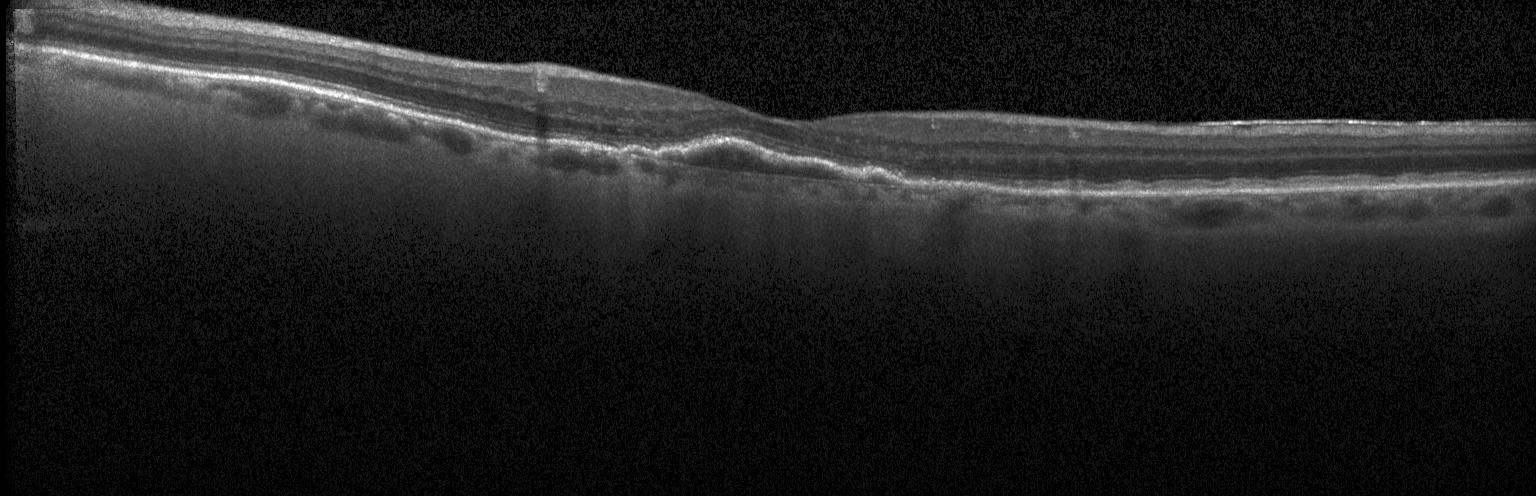

OCT finding: a choroidal neovascular membrane.